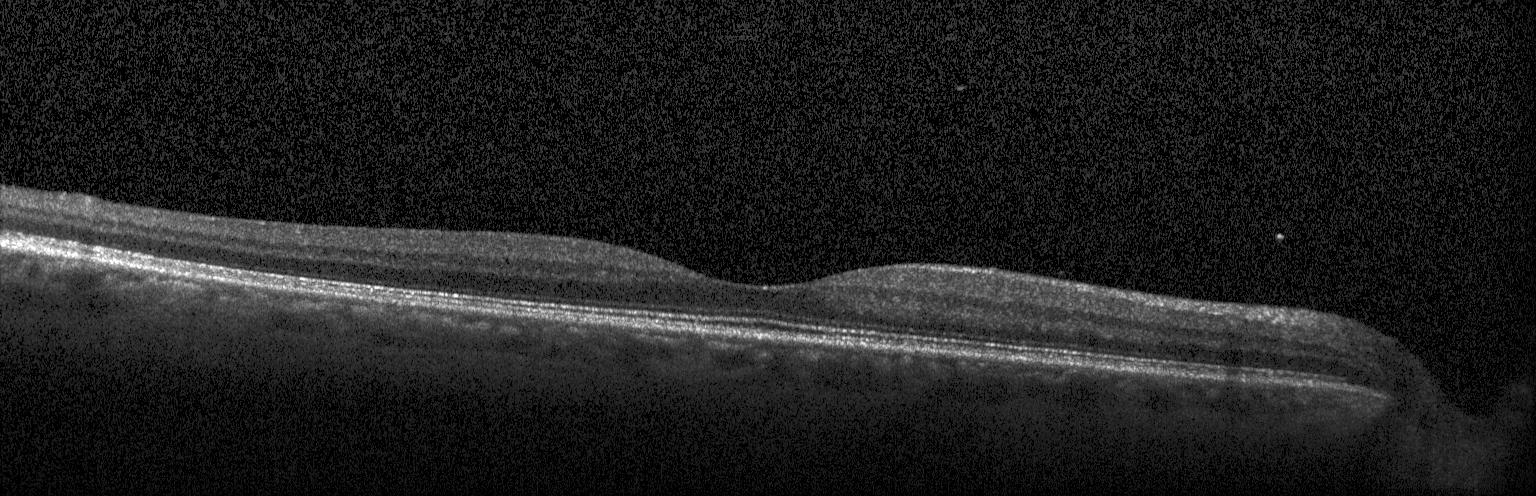 OCT line scan — Assessment: no choroidal neovascularization, diabetic macular edema, or drusen.